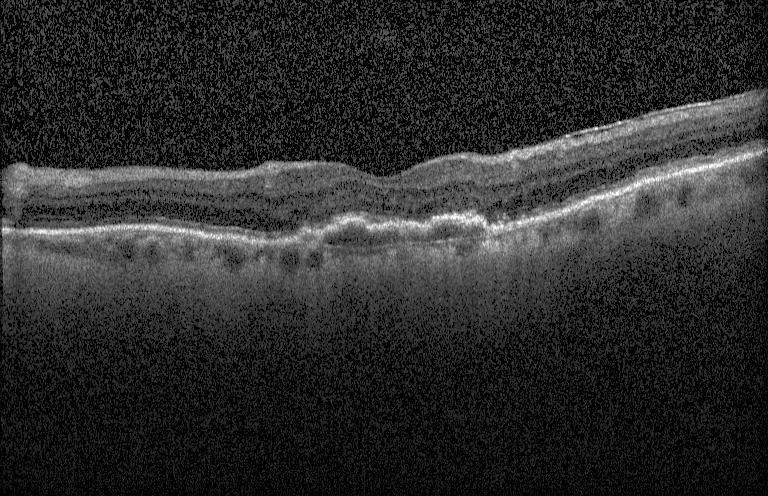 Optical coherence tomography B-scan — Impression: a choroidal neovascular membrane.